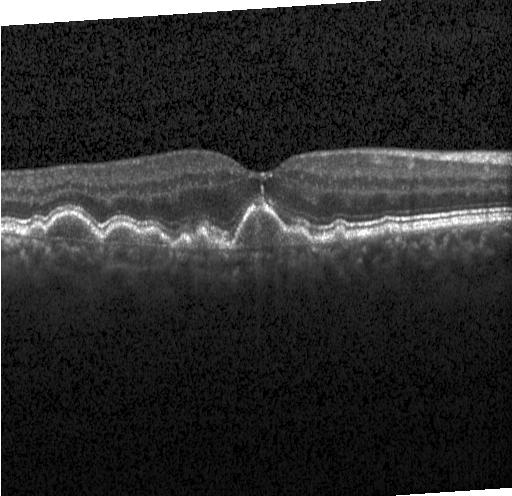
Optical coherence tomography B-scan.
Macular OCT: drusen.